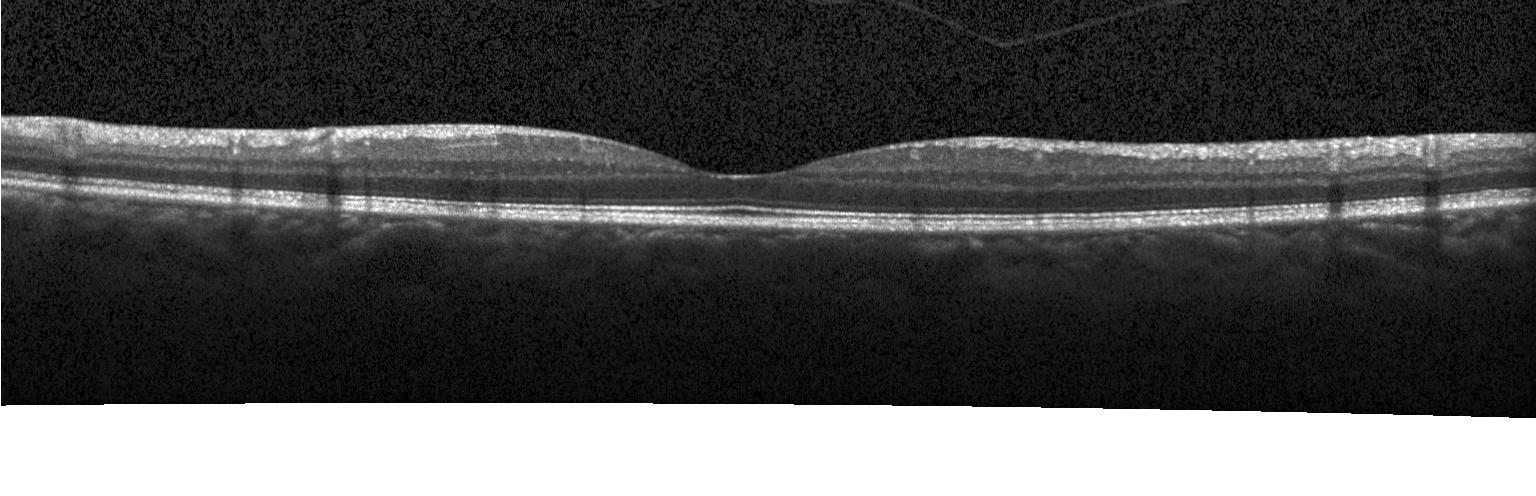 Macular OCT: neither choroidal neovascularization, diabetic macular edema, nor drusen.